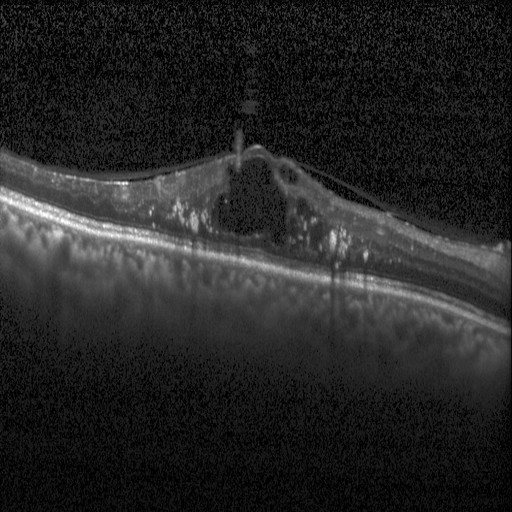

Retinal OCT B-scan; spectral-domain optical coherence tomography; centered on the fovea; acquired on a Heidelberg Spectralis.
Impression: diabetic macular edema (DME).